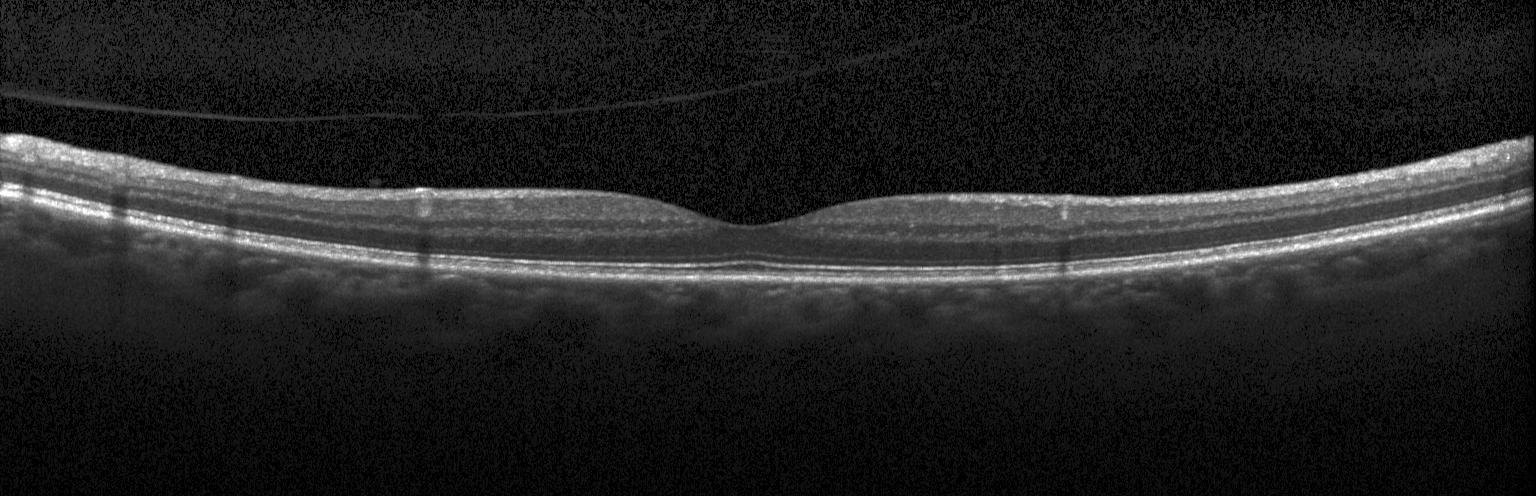 Diagnosis: neither choroidal neovascularization, diabetic macular edema, nor drusen.